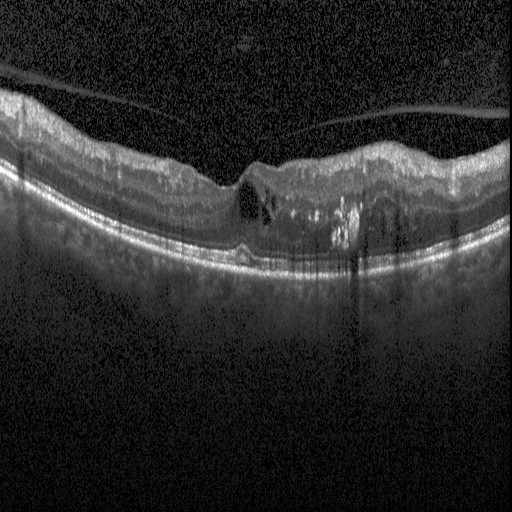

Spectral-domain OCT B-scan: DME.